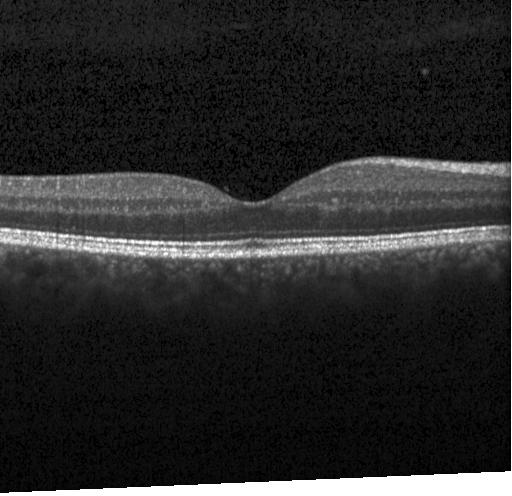
OCT B-scan showing neither CNV, DME, nor drusen.